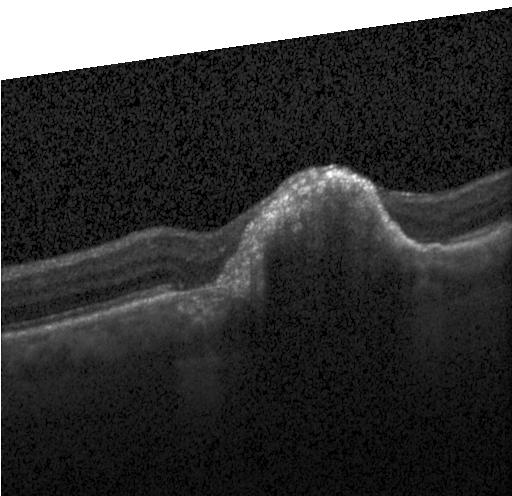 SD-OCT · acquired on a Heidelberg Spectralis · retinal OCT cross-section
OCT finding: CNV.